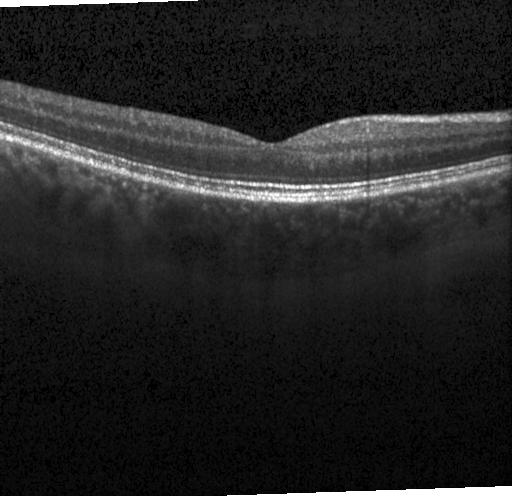

OCT B-scan, fovea-centered, spectral-domain OCT. Finding: no choroidal neovascularization, no diabetic macular edema, and no drusen.